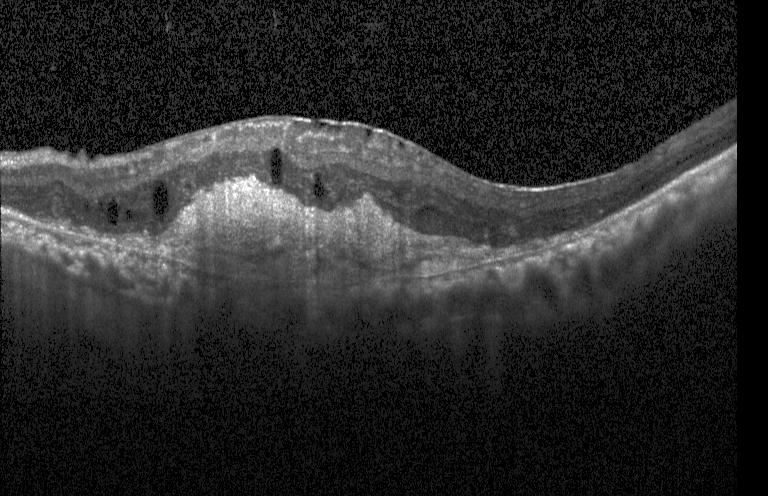 Retinal OCT cross-section.
This B-scan demonstrates a choroidal neovascular membrane.